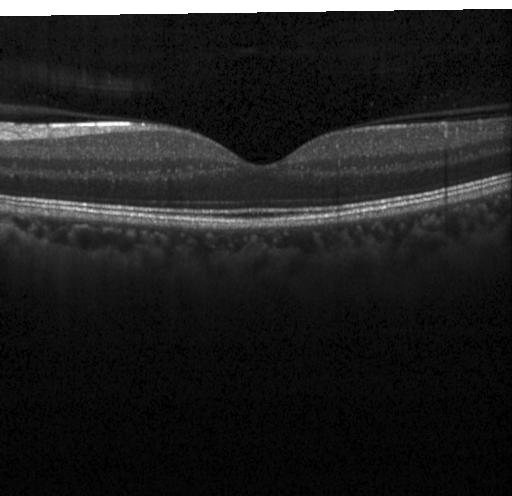
Macular OCT: neither choroidal neovascularization, diabetic macular edema, nor drusen.